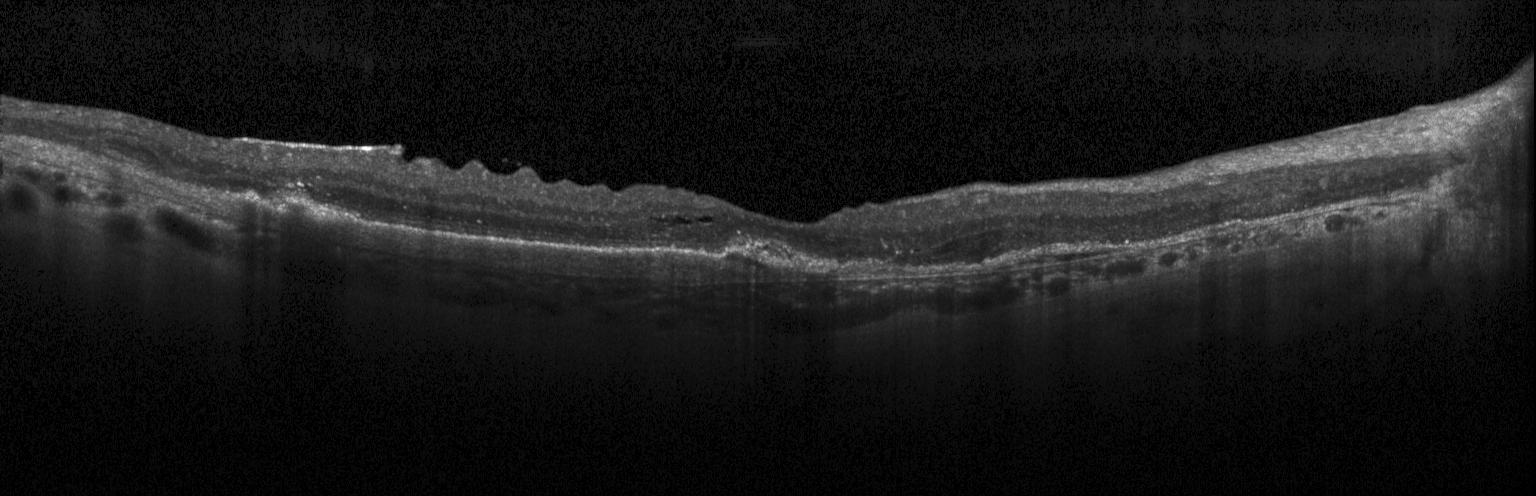

Spectral-domain optical coherence tomography. Retinal OCT B-scan. Centered on the fovea.
Finding: choroidal neovascularization (CNV).